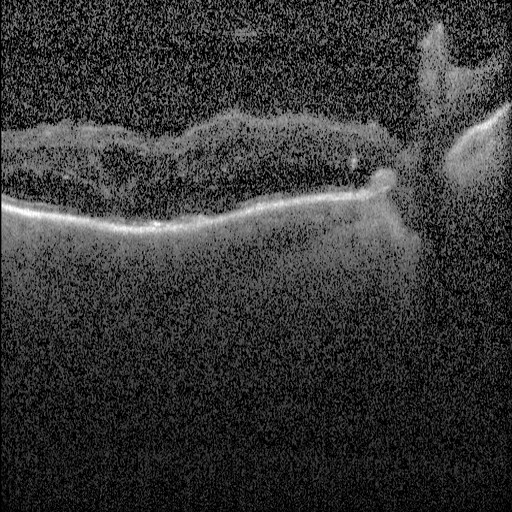

Diabetic macular edema.